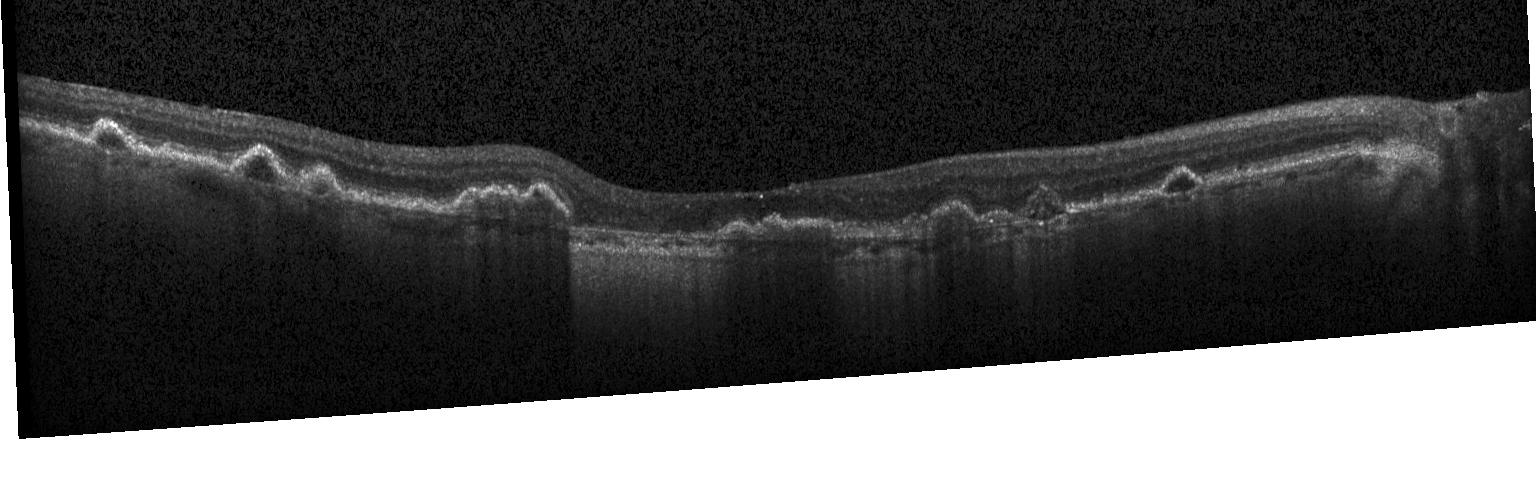
Retinal OCT cross-section.
Impression: choroidal neovascularization.